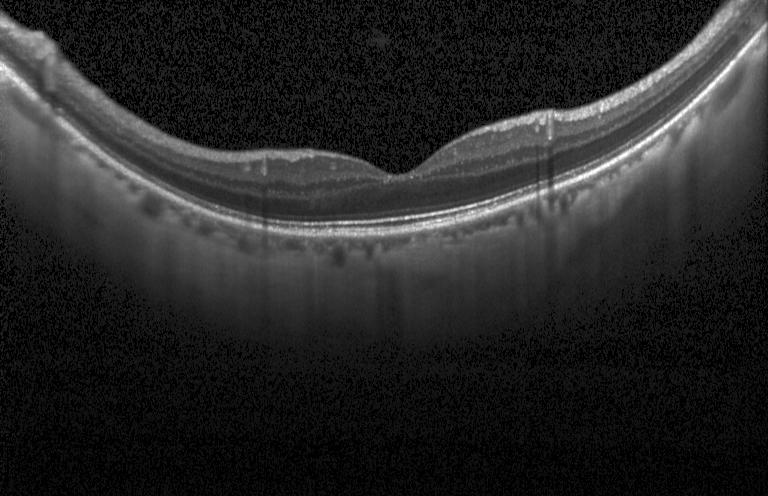
Optical coherence tomography scan
Dx: no evidence of choroidal neovascularization, diabetic macular edema, or drusen.